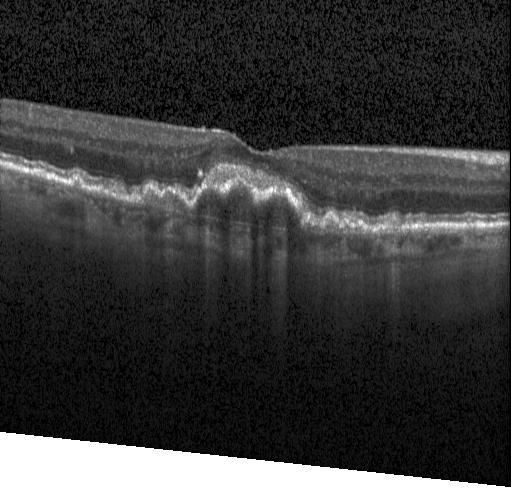
Finding: a choroidal neovascular membrane.